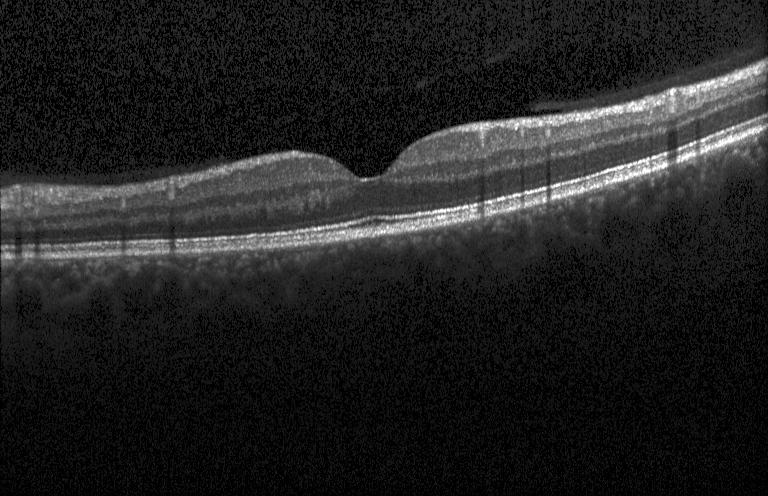 Optical coherence tomography scan. Acquired on a Heidelberg Spectralis. Spectral-domain optical coherence tomography
Finding: no CNV, no DME, and no drusen.